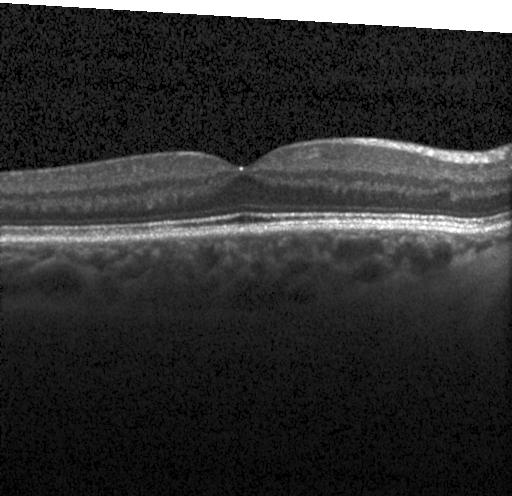 Through the macula, OCT B-scan. Macular OCT: no choroidal neovascularization, no diabetic macular edema, and no drusen.